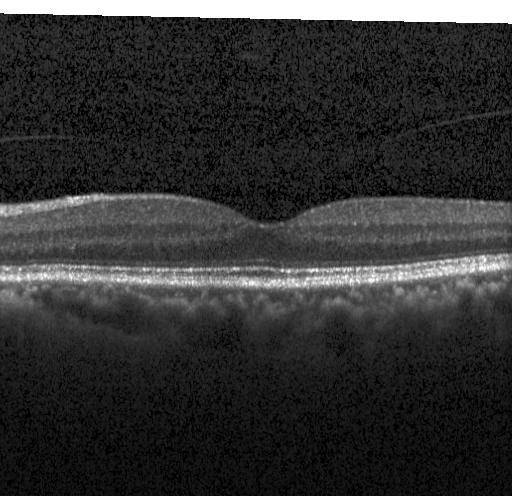 Dx: no evidence of choroidal neovascularization, diabetic macular edema, or drusen.